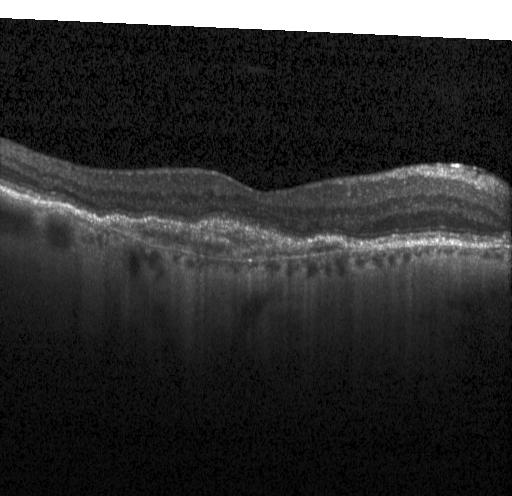
Retinal OCT cross-section
The scan shows a choroidal neovascular membrane.